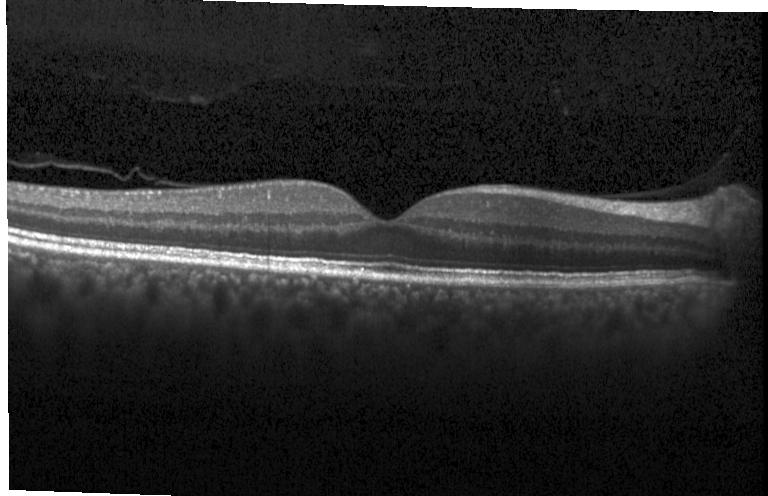 Optical coherence tomography scan · instrument: Heidelberg Spectralis · macular scan — Diagnosis: no CNV, no DME, and no drusen.